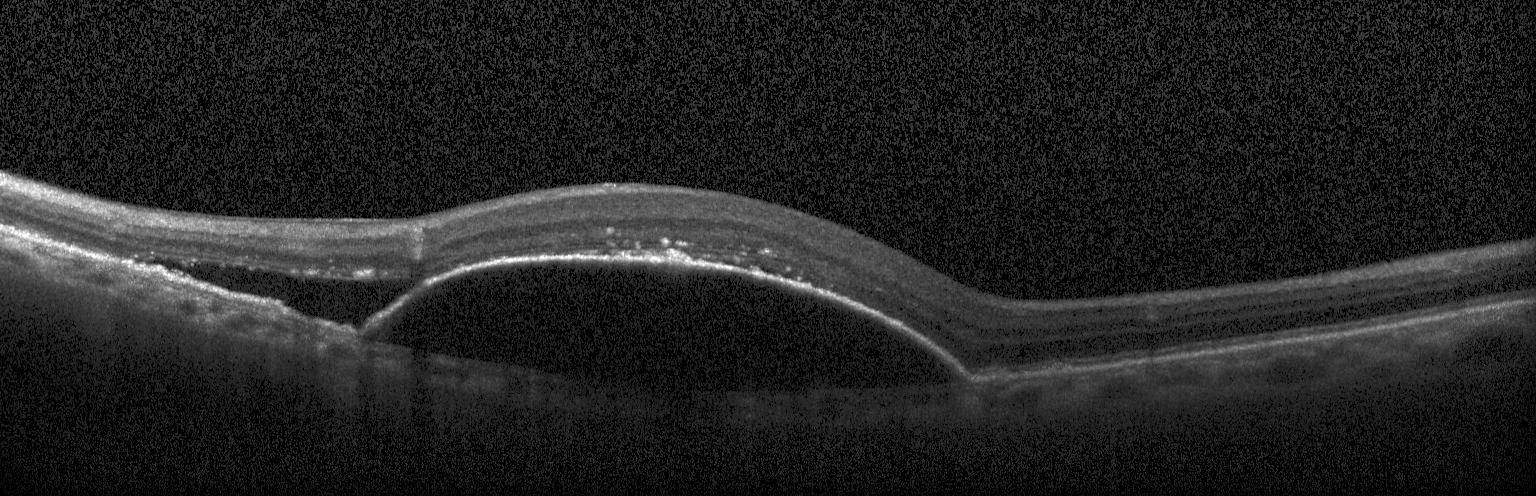 OCT line scan — Impression: choroidal neovascularization (CNV).